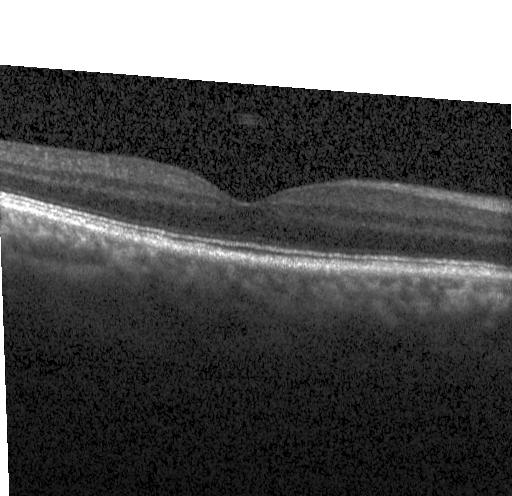
OCT B-scan. Heidelberg Spectralis OCT system — This B-scan demonstrates neither choroidal neovascularization, diabetic macular edema, nor drusen.